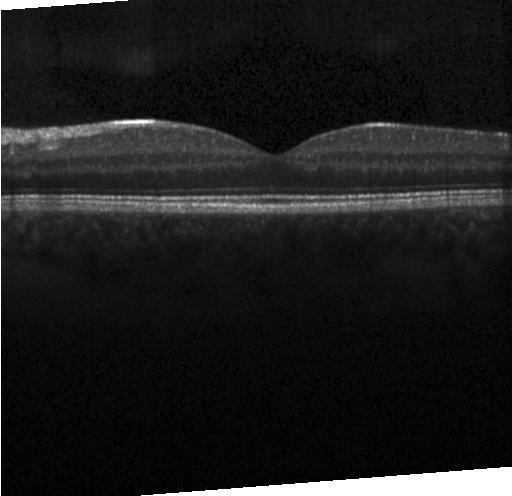

Retinal OCT B-scan · instrument: Heidelberg Spectralis · SD-OCT · centered on the fovea. Assessment: no evidence of CNV, DME, or drusen.